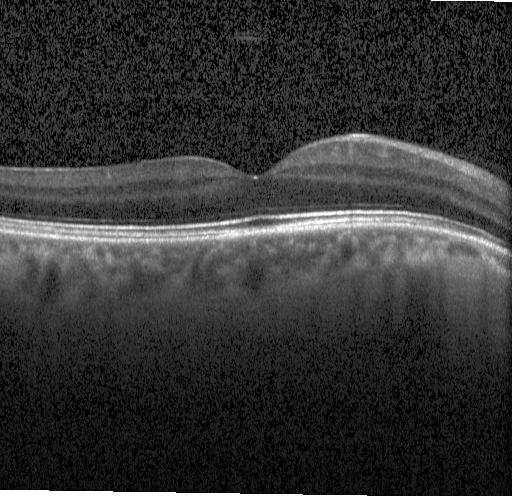
Heidelberg Spectralis OCT system · OCT line scan · spectral-domain OCT · macular scan — No choroidal neovascularization, no diabetic macular edema, and no drusen.